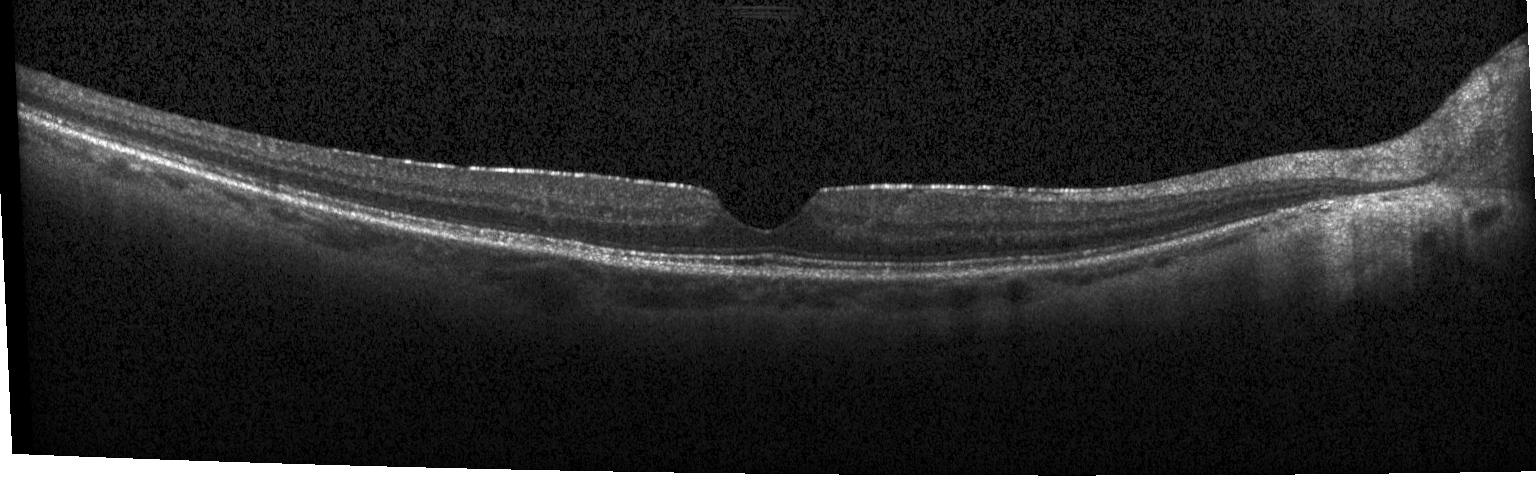

Centered on the fovea, retinal OCT B-scan, Heidelberg Spectralis OCT system.
Diagnosis: neither choroidal neovascularization, diabetic macular edema, nor drusen.